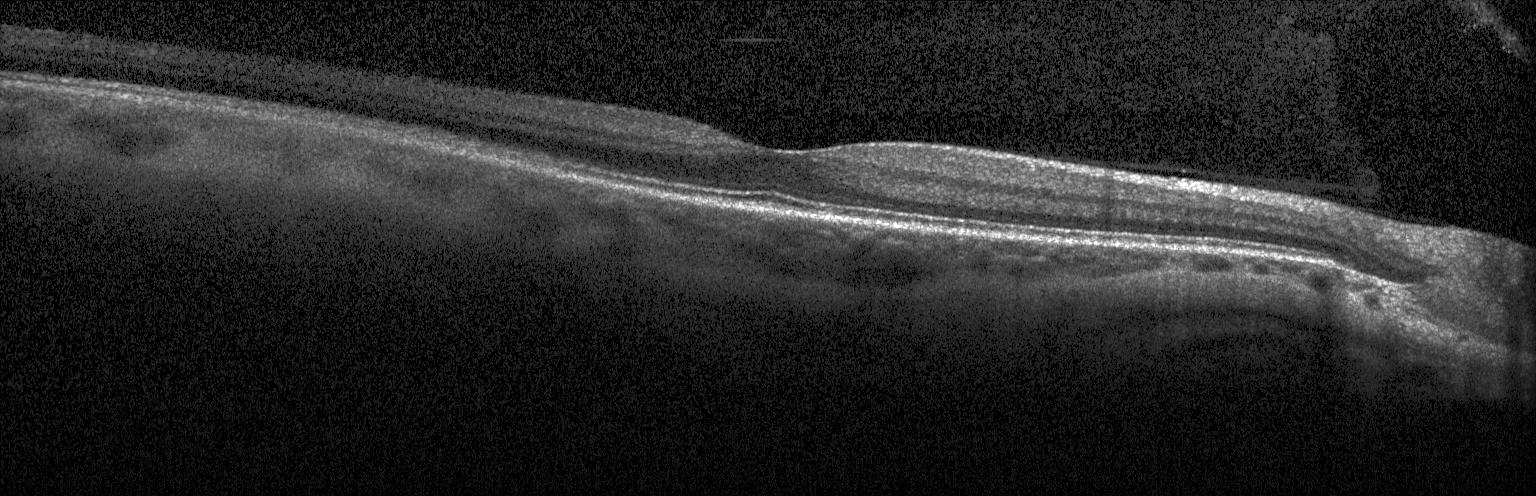

Assessment: no CNV, DME, or drusen.